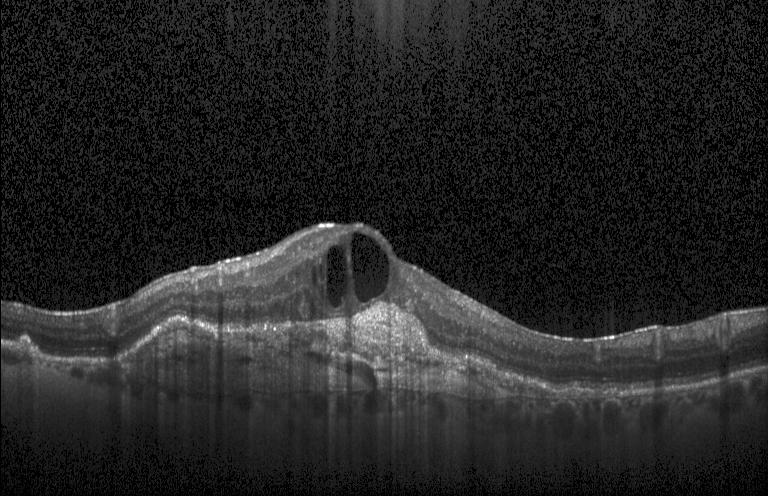
Spectral-domain optical coherence tomography; retinal OCT cross-section.
Diagnosis: choroidal neovascularization.